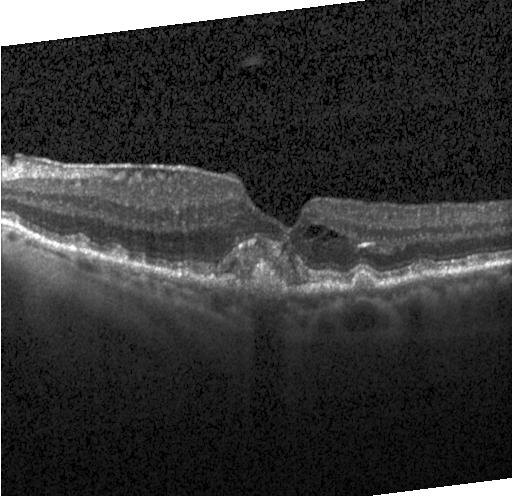
Spectral-domain optical coherence tomography. OCT line scan. Acquired on a Heidelberg Spectralis. Horizontal scan through the fovea.
Assessment: a choroidal neovascular membrane.